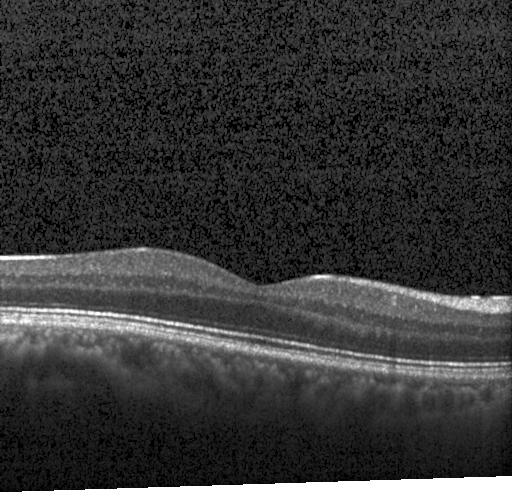 Spectral-domain optical coherence tomography; retinal OCT B-scan; Heidelberg Spectralis OCT system.
This B-scan demonstrates no evidence of CNV, DME, or drusen.